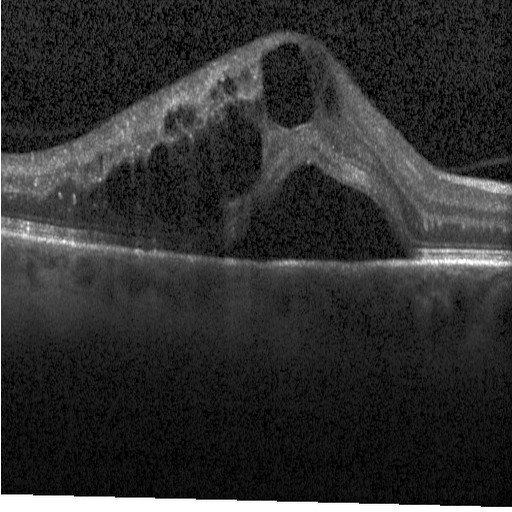

Instrument: Heidelberg Spectralis. Through the macula. Optical coherence tomography B-scan. Spectral-domain OCT. This B-scan demonstrates diabetic macular edema.